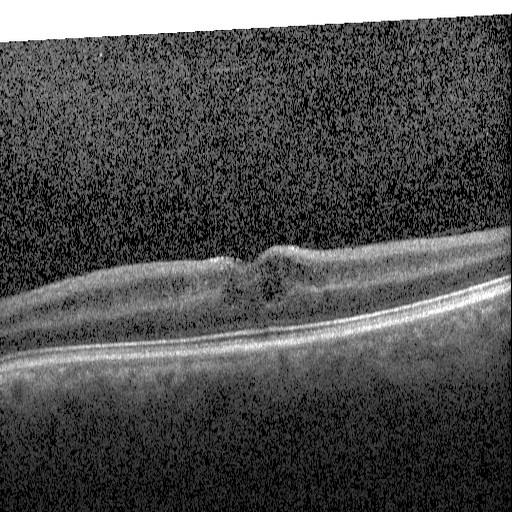
Optical coherence tomography scan · centered on the fovea · SD-OCT · Heidelberg Spectralis — Impression: diabetic macular edema.